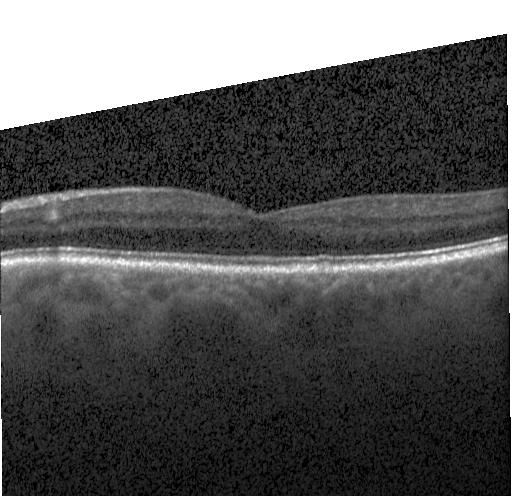

Diagnosis: no choroidal neovascularization, diabetic macular edema, or drusen.